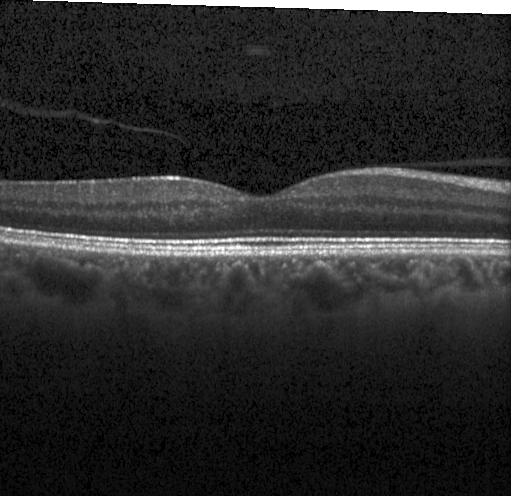
Spectral-domain OCT. OCT line scan. Through the macula
Macular OCT: neither choroidal neovascularization, diabetic macular edema, nor drusen.